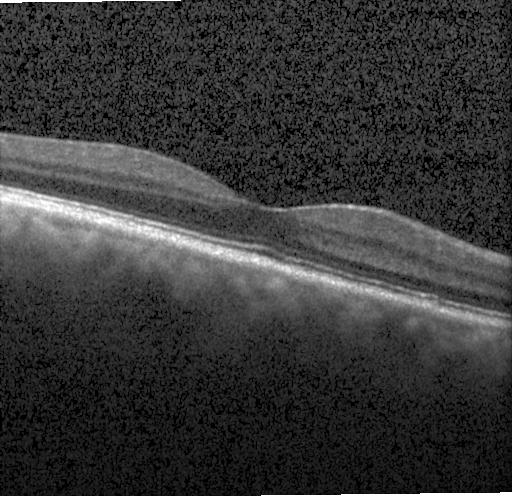

Assessment: no CNV, DME, or drusen.